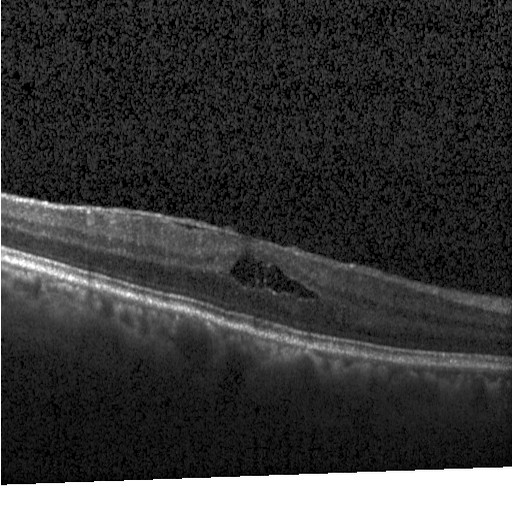

Macular OCT: diabetic macular edema.